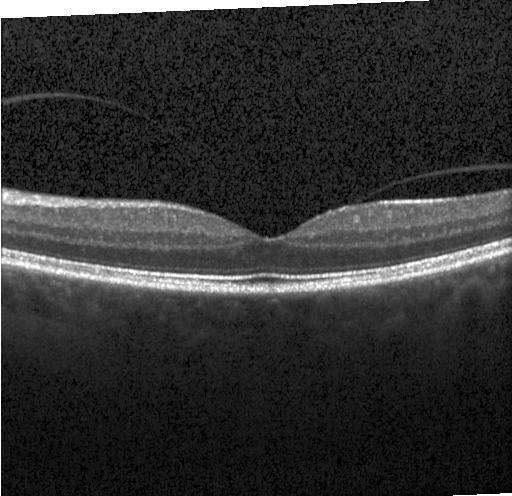

Retinal OCT cross-section; spectral-domain optical coherence tomography — Assessment: no choroidal neovascularization, no diabetic macular edema, and no drusen.